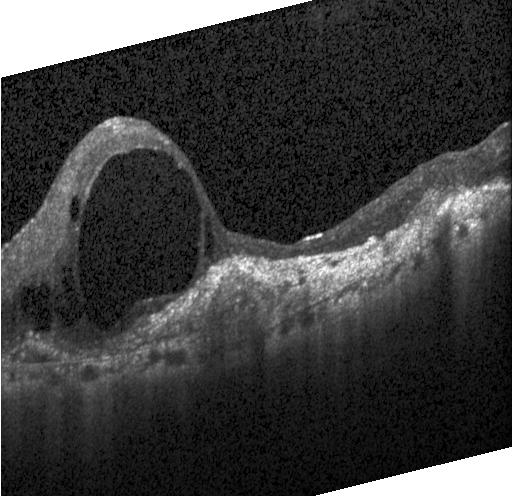

Finding: a choroidal neovascular membrane.